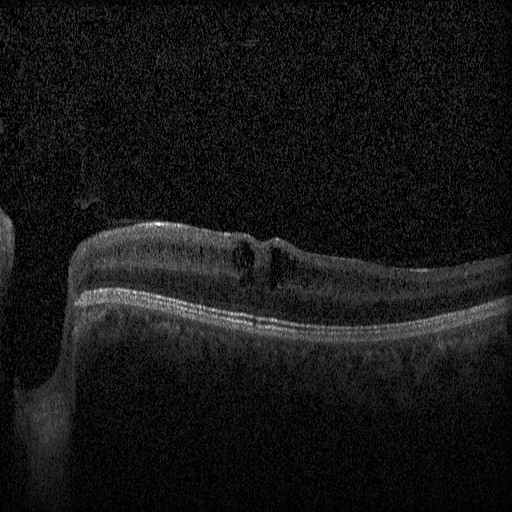

OCT scan showing DME.